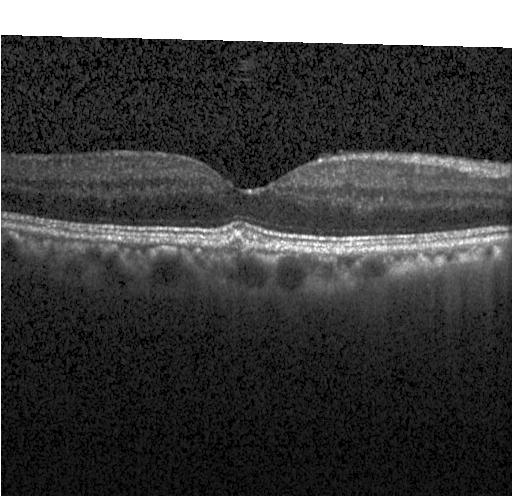

OCT line scan — This B-scan demonstrates no evidence of choroidal neovascularization, diabetic macular edema, or drusen.